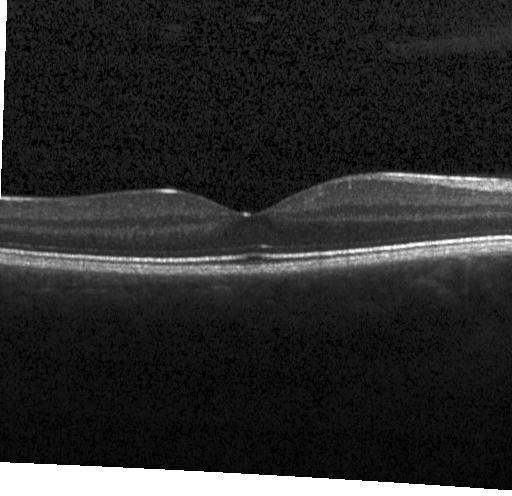 Fovea-centered, retinal OCT cross-section, spectral-domain optical coherence tomography, acquired on a Heidelberg Spectralis
No choroidal neovascularization, diabetic macular edema, or drusen.